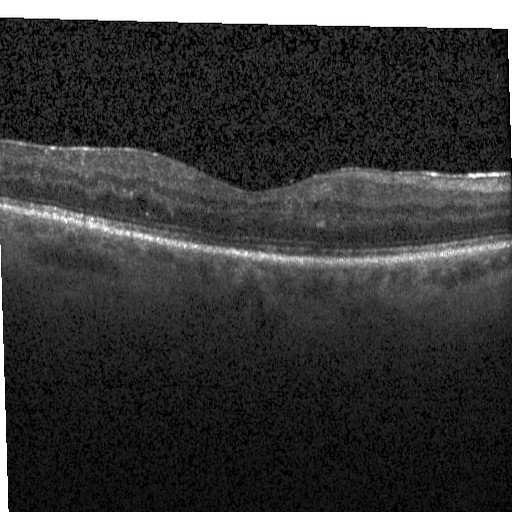
Assessment: diabetic macular edema.